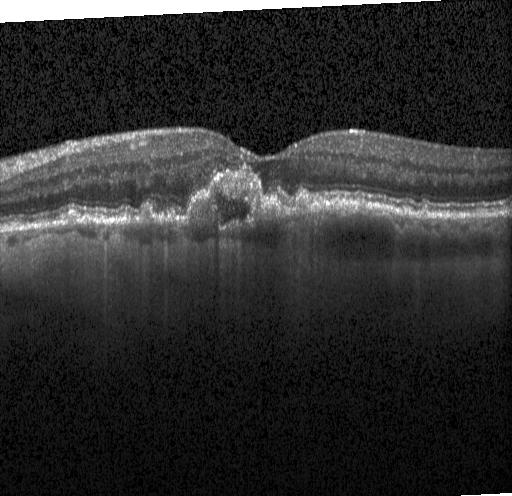
Optical coherence tomography B-scan · horizontal scan through the fovea · Heidelberg Spectralis.
Impression: choroidal neovascularization.